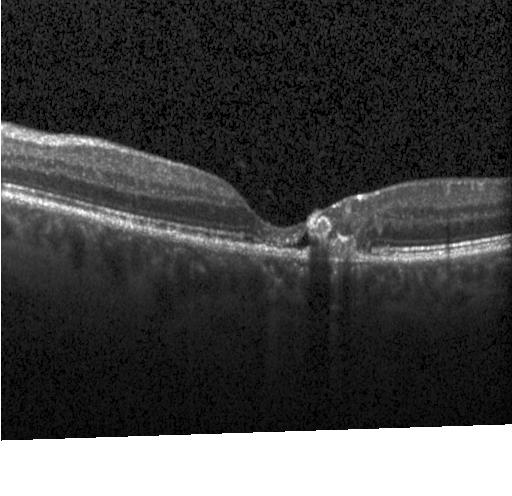

Dx: CNV.